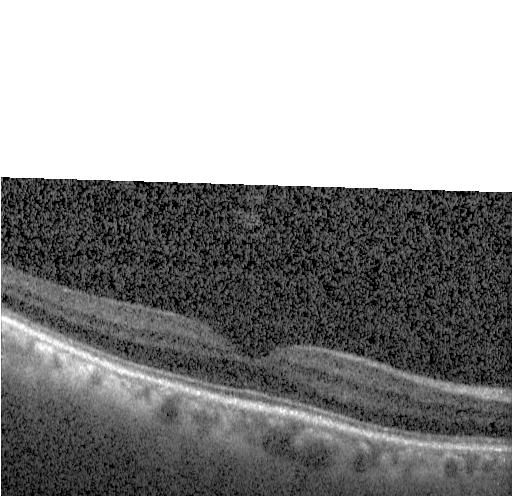
Retinal OCT cross-section.
No choroidal neovascularization, no diabetic macular edema, and no drusen.